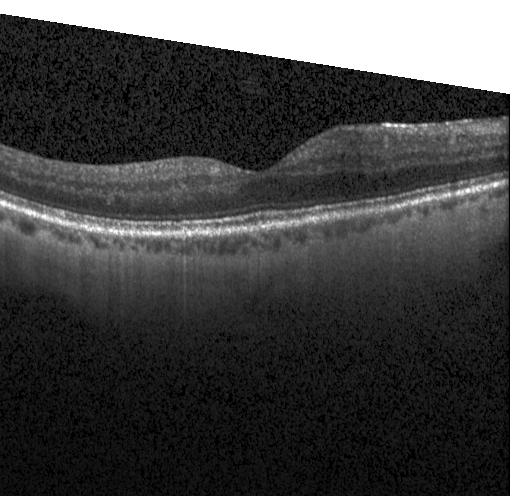

OCT line scan; instrument: Heidelberg Spectralis; SD-OCT; centered on the fovea. Finding: no evidence of choroidal neovascularization, diabetic macular edema, or drusen.